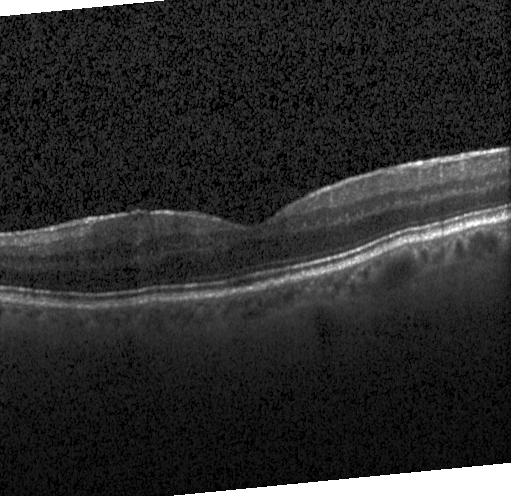

Macular OCT: no choroidal neovascularization, no diabetic macular edema, and no drusen.